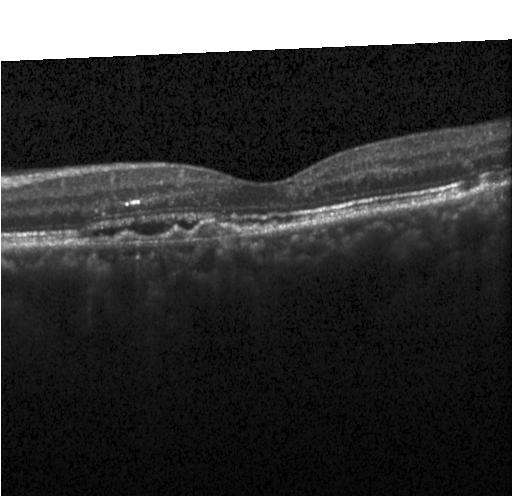

OCT line scan — Finding: CNV.